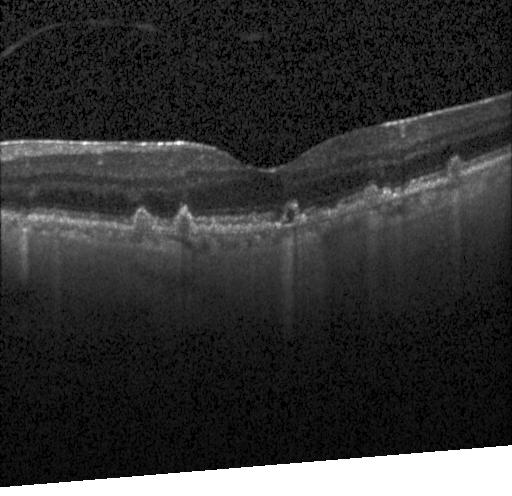

Diagnosis: drusen.